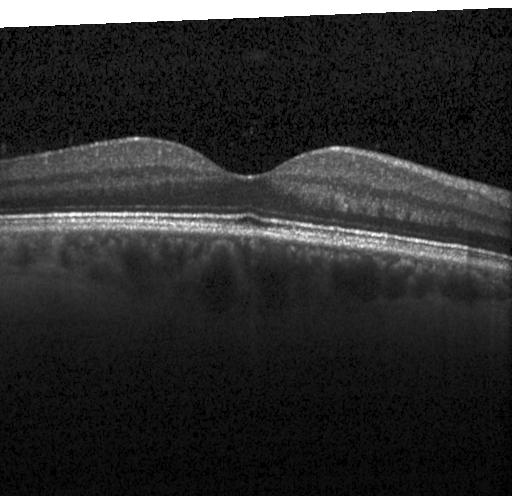
Optical coherence tomography scan. Instrument: Heidelberg Spectralis. Spectral-domain optical coherence tomography. Diagnosis: no choroidal neovascularization, diabetic macular edema, or drusen.